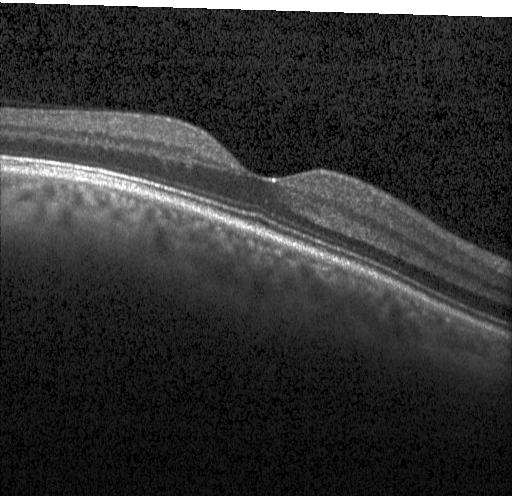

OCT line scan — Finding: no choroidal neovascularization, no diabetic macular edema, and no drusen.